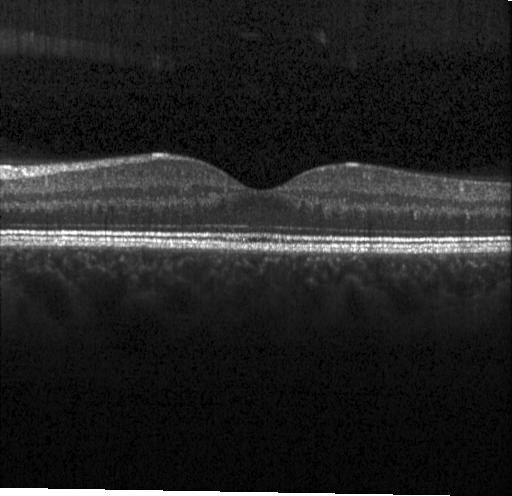 Acquired on a Heidelberg Spectralis · SD-OCT · optical coherence tomography B-scan. This B-scan demonstrates no CNV, no DME, and no drusen.